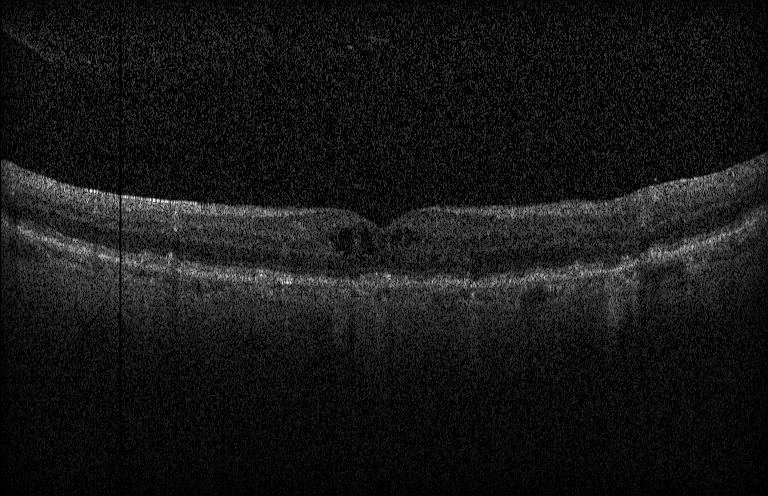 Spectral-domain OCT. Centered on the fovea. Heidelberg Spectralis OCT system. Optical coherence tomography scan.
The scan shows choroidal neovascularization (CNV).